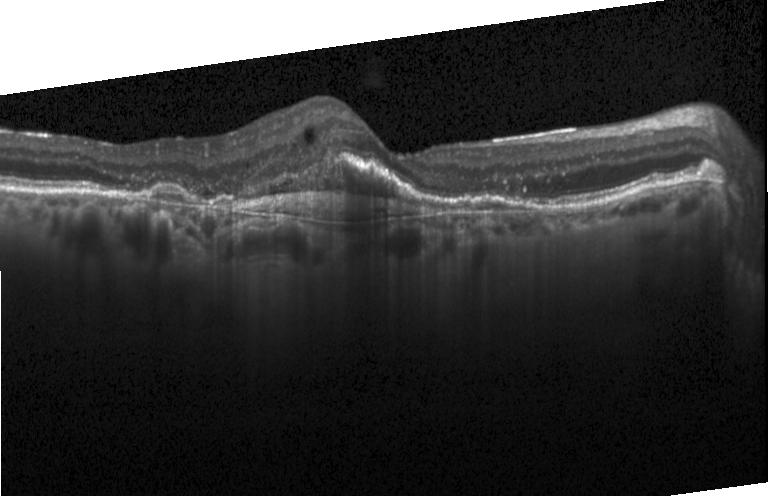 Retinal OCT B-scan
Assessment: CNV.